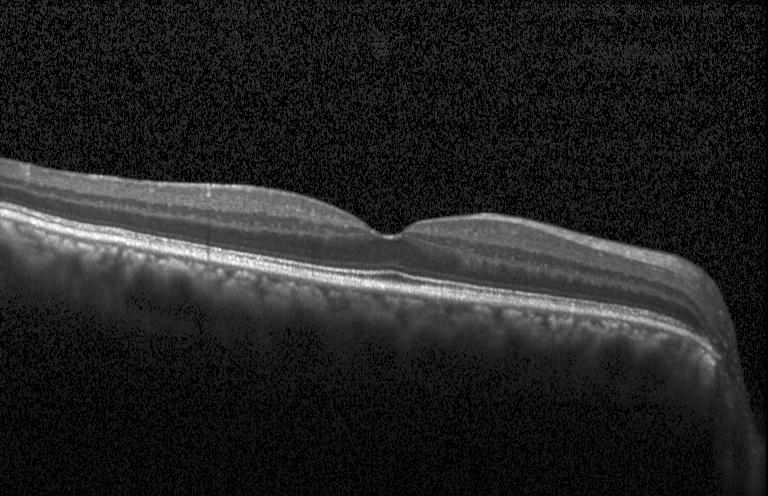 Spectral-domain OCT. Macular scan. Retinal OCT B-scan. Diagnosis: no CNV, DME, or drusen.